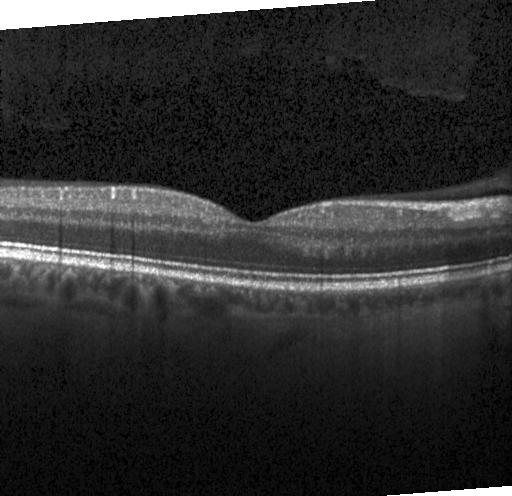 Spectral-domain optical coherence tomography · through the macula · OCT line scan · Heidelberg Spectralis. Finding: no choroidal neovascularization, diabetic macular edema, or drusen.